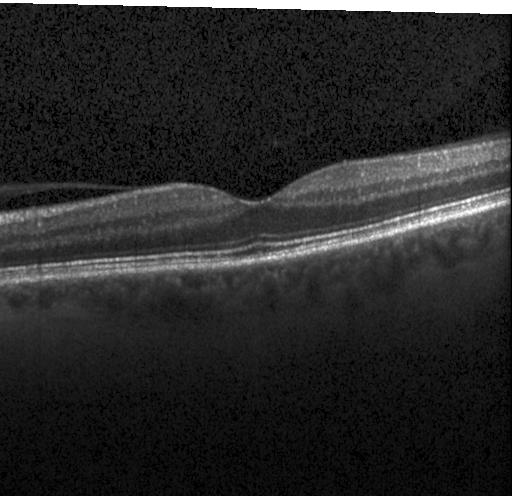
Acquired on a Heidelberg Spectralis. OCT B-scan. Diagnosis: no evidence of choroidal neovascularization, diabetic macular edema, or drusen.